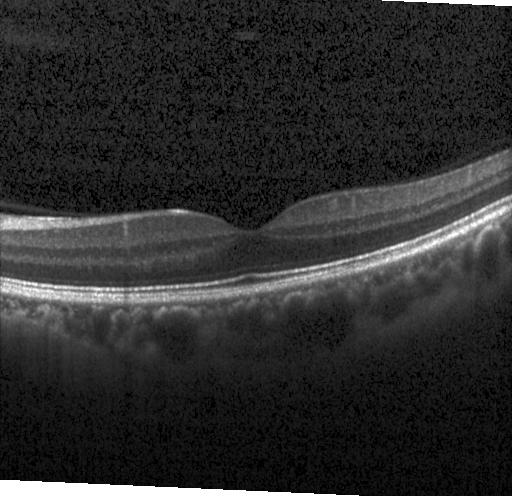 Horizontal scan through the fovea, Heidelberg Spectralis OCT system, optical coherence tomography B-scan — Finding: neither CNV, DME, nor drusen.